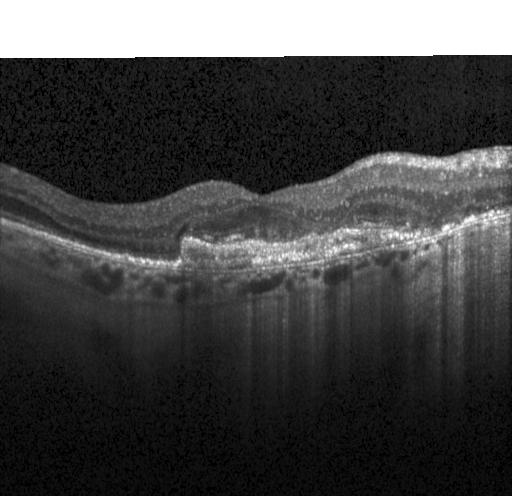
Spectral-domain OCT B-scan: a choroidal neovascular membrane.